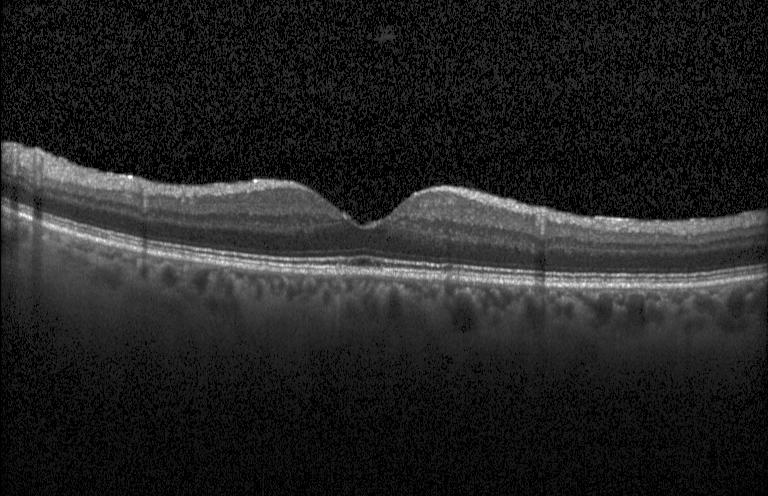 Retinal OCT cross-section
Dx: no CNV, DME, or drusen.